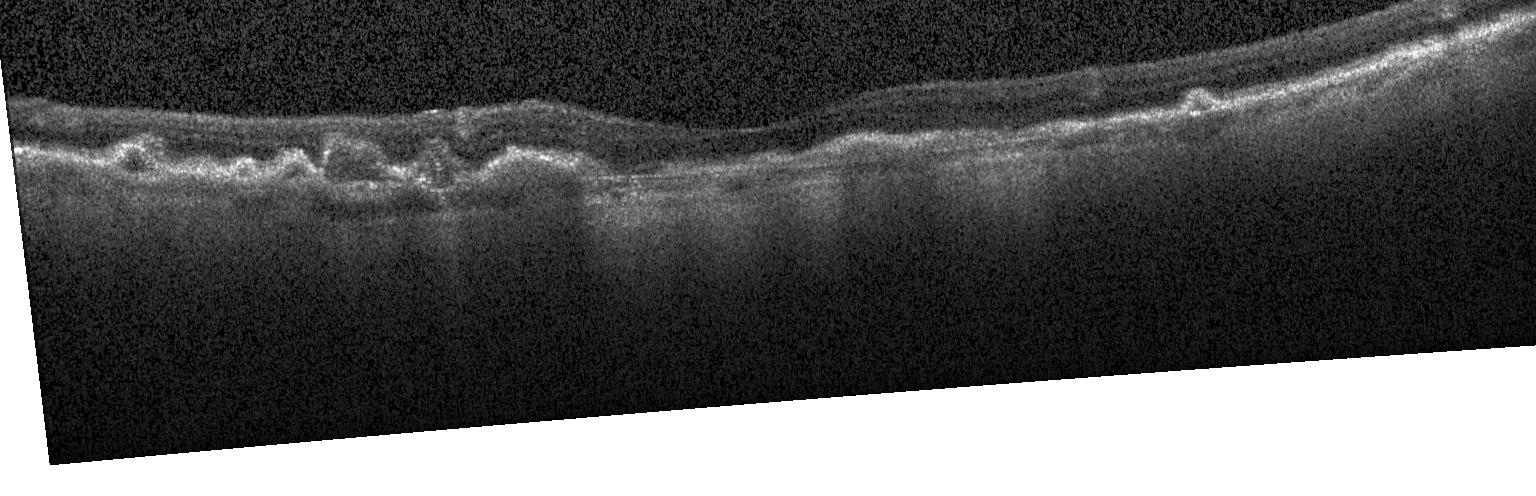 Finding: a choroidal neovascular membrane.